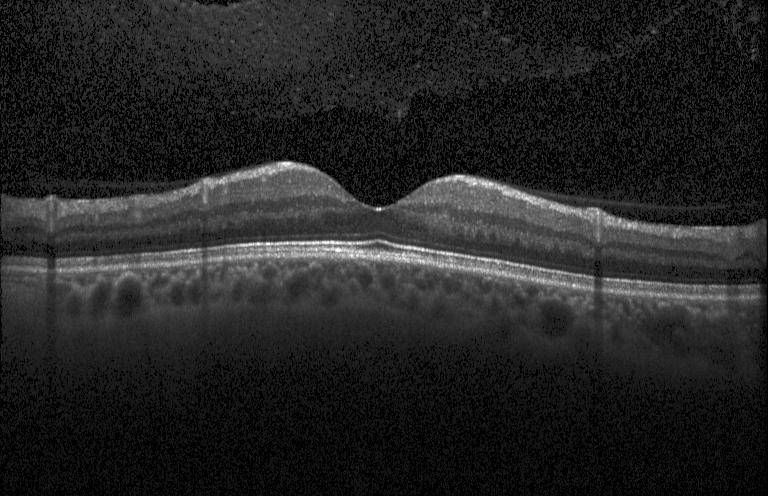
Macular scan, optical coherence tomography scan, SD-OCT
Impression: no evidence of choroidal neovascularization, diabetic macular edema, or drusen.